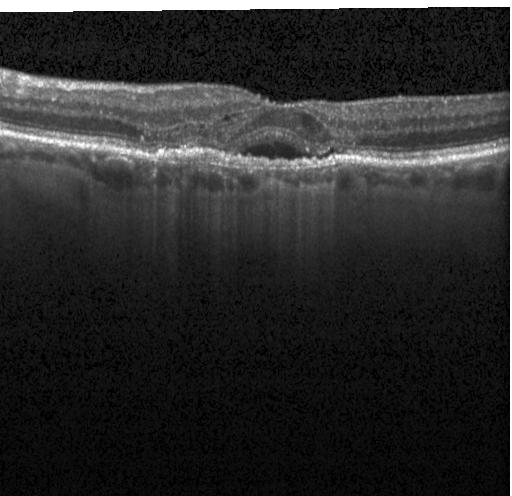 Impression: choroidal neovascularization (CNV).